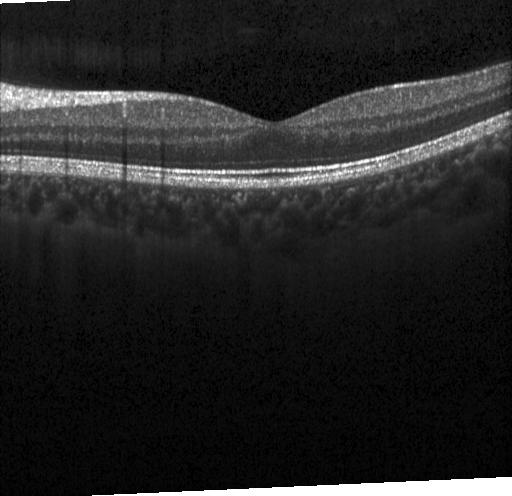 Acquired on a Heidelberg Spectralis. OCT B-scan. Through the macula — This B-scan demonstrates neither CNV, DME, nor drusen.